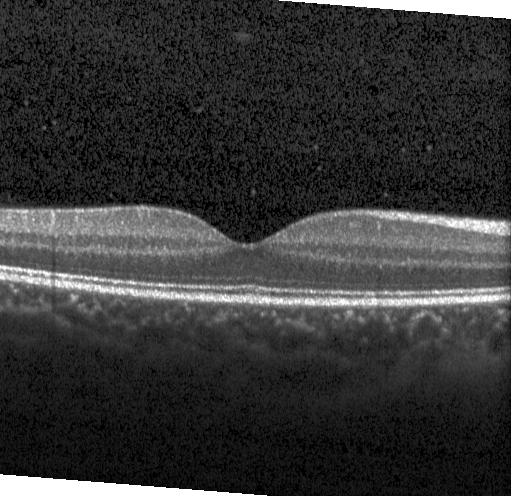 OCT finding: no CNV, no DME, and no drusen.